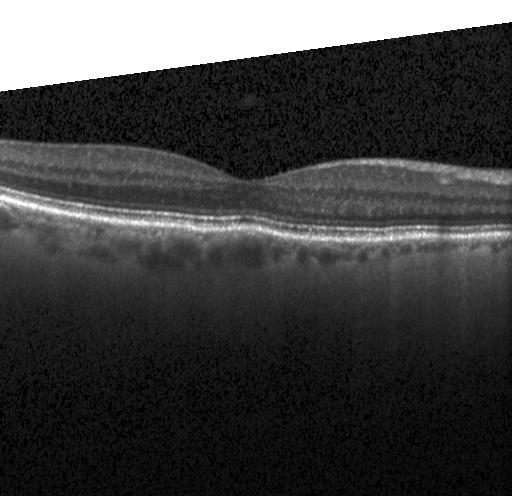 Macular OCT: no evidence of CNV, DME, or drusen.